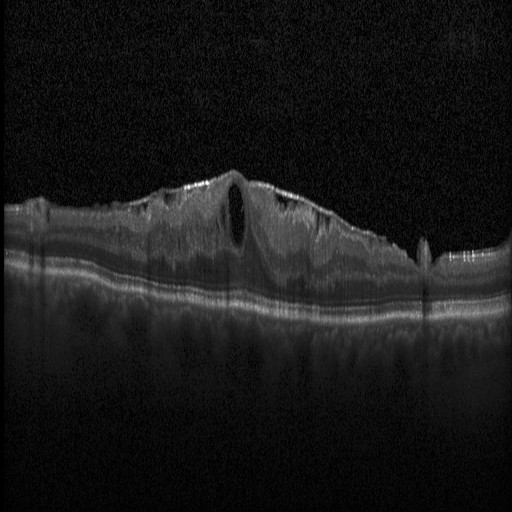

OCT B-scan · fovea-centered · instrument: Heidelberg Spectralis. Finding: diabetic macular edema (DME).